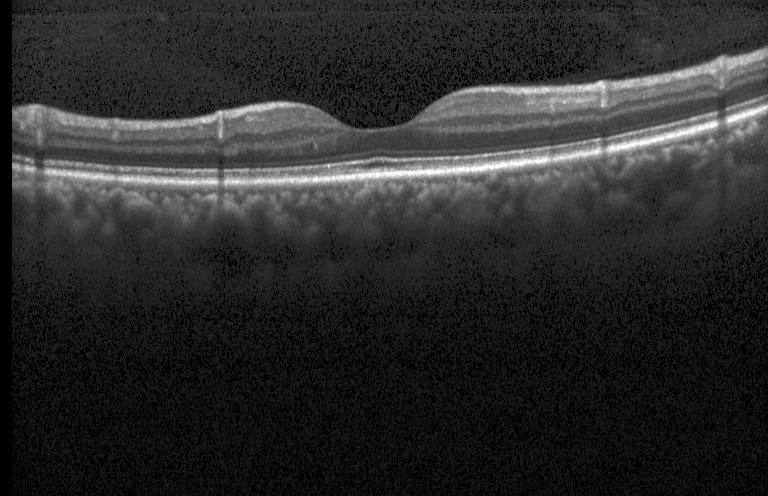
Retinal OCT cross-section; acquired on a Heidelberg Spectralis — Macular OCT: neither CNV, DME, nor drusen.